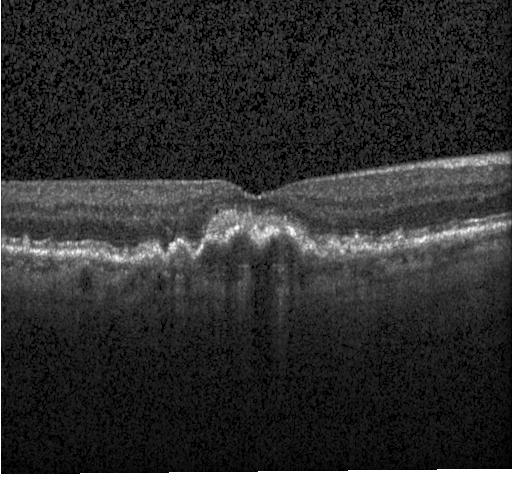

Heidelberg Spectralis; optical coherence tomography B-scan. A choroidal neovascular membrane.